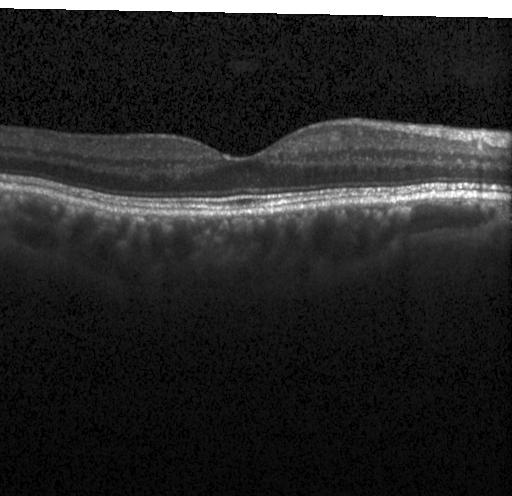
Impression: no evidence of CNV, DME, or drusen.